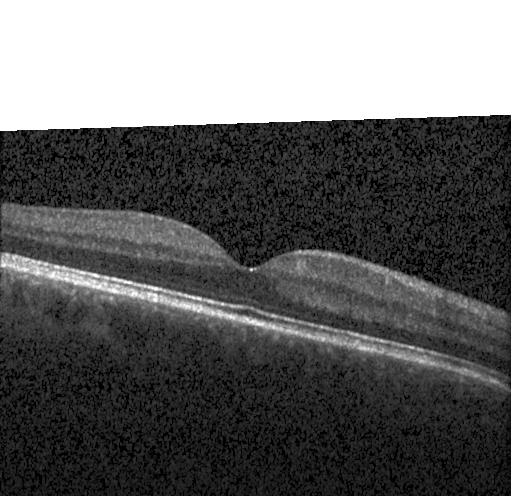

Macular OCT demonstrating neither choroidal neovascularization, diabetic macular edema, nor drusen.